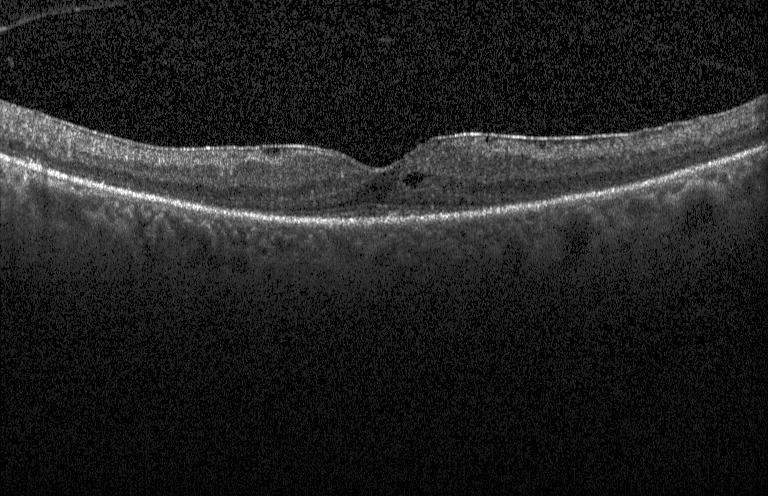 OCT scan showing DME.